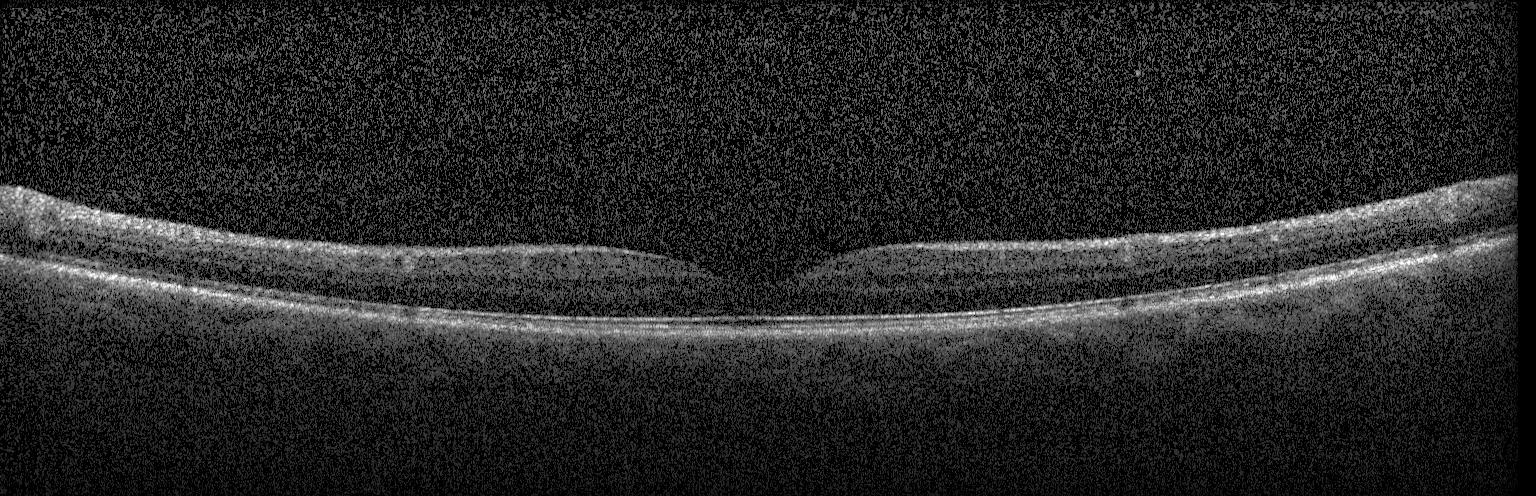 Spectral-domain optical coherence tomography. OCT line scan. Diagnosis: neither CNV, DME, nor drusen.